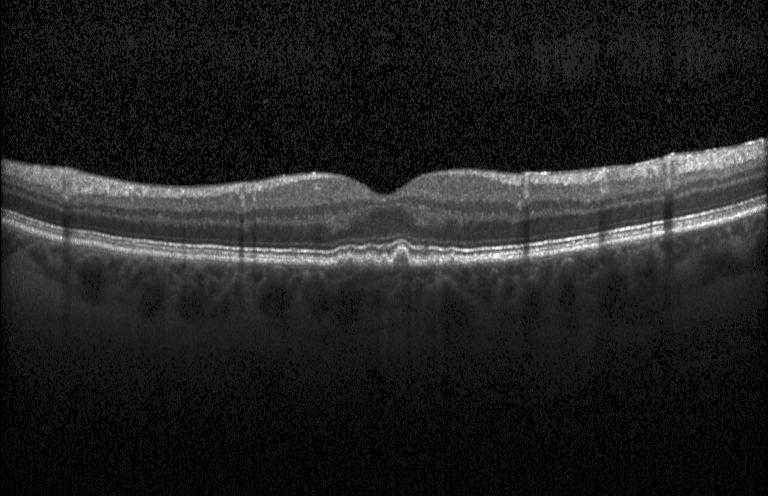
Centered on the fovea; OCT line scan; Heidelberg Spectralis — Finding: sub-RPE drusenoid deposits.